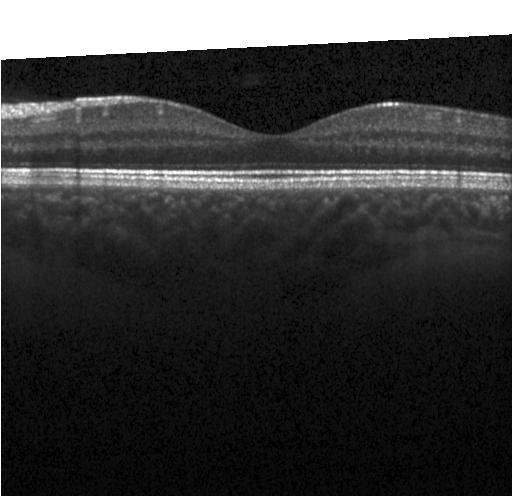

Heidelberg Spectralis OCT system · spectral-domain OCT · optical coherence tomography scan · horizontal scan through the fovea
Diagnosis: no CNV, DME, or drusen.